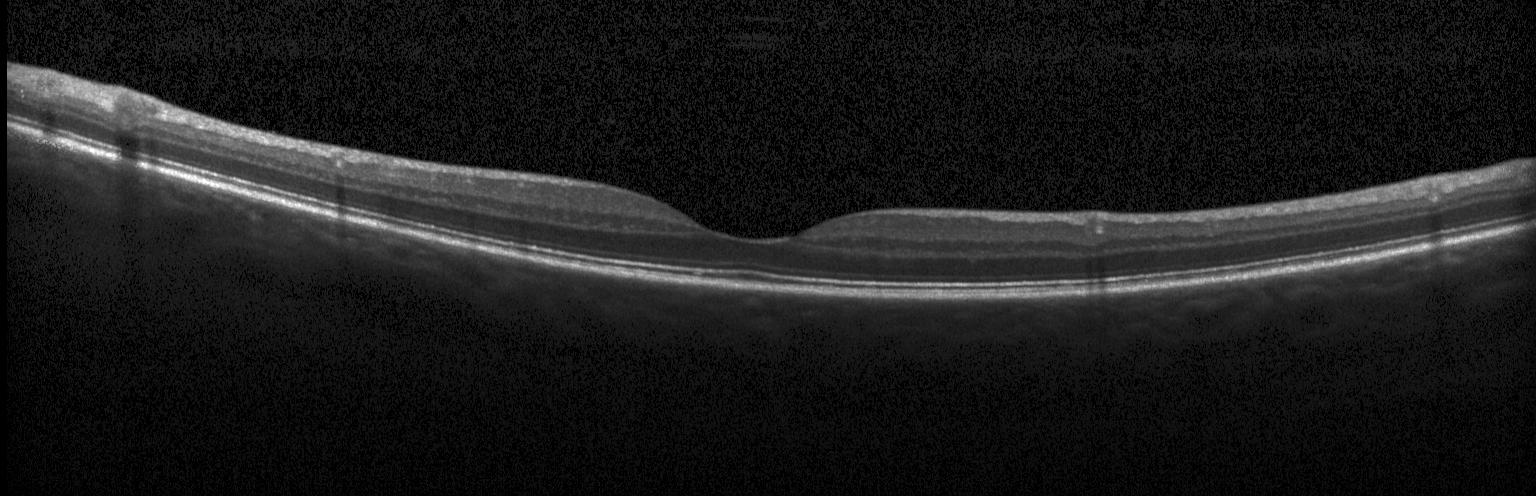
Diagnosis: no evidence of choroidal neovascularization, diabetic macular edema, or drusen.